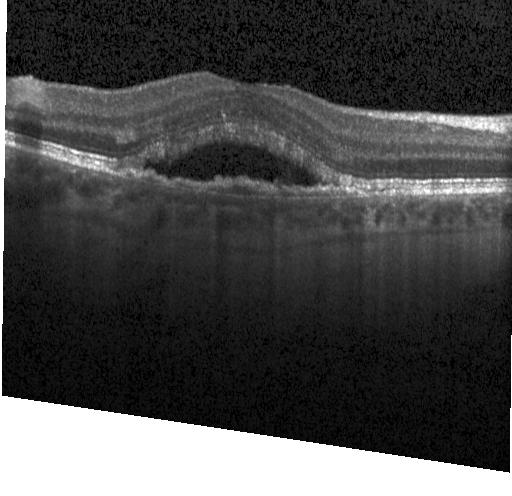 Finding: a choroidal neovascular membrane.